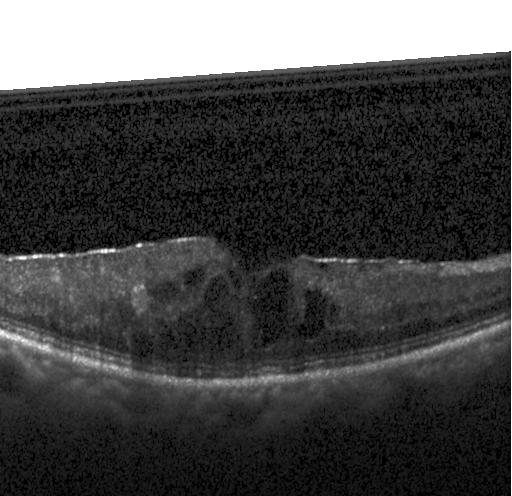
OCT B-scan. Diagnosis: DME.